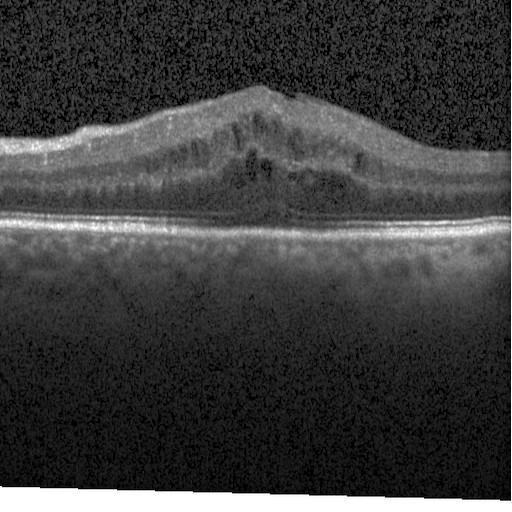 Optical coherence tomography B-scan.
Assessment: DME.